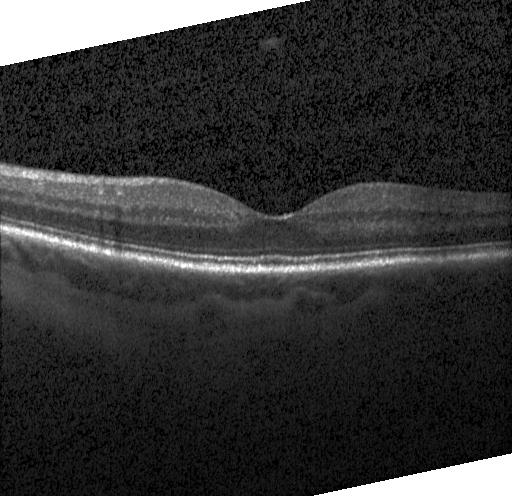
Retinal OCT cross-section; Heidelberg Spectralis
Impression: no choroidal neovascularization, diabetic macular edema, or drusen.